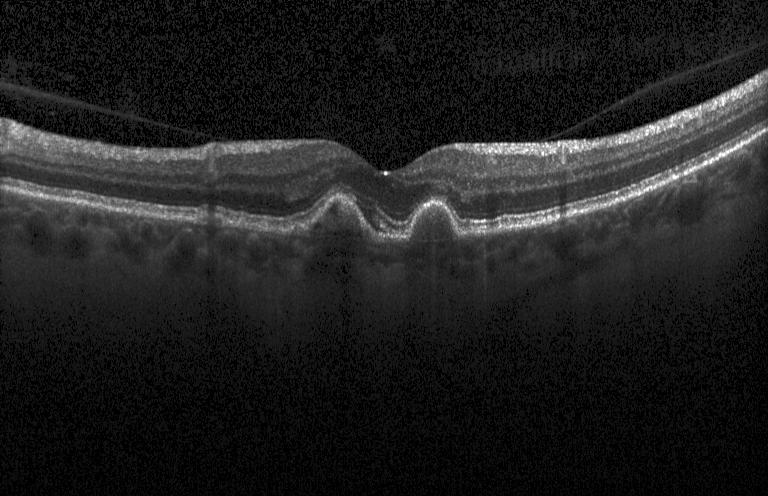 Assessment: sub-RPE drusenoid deposits.